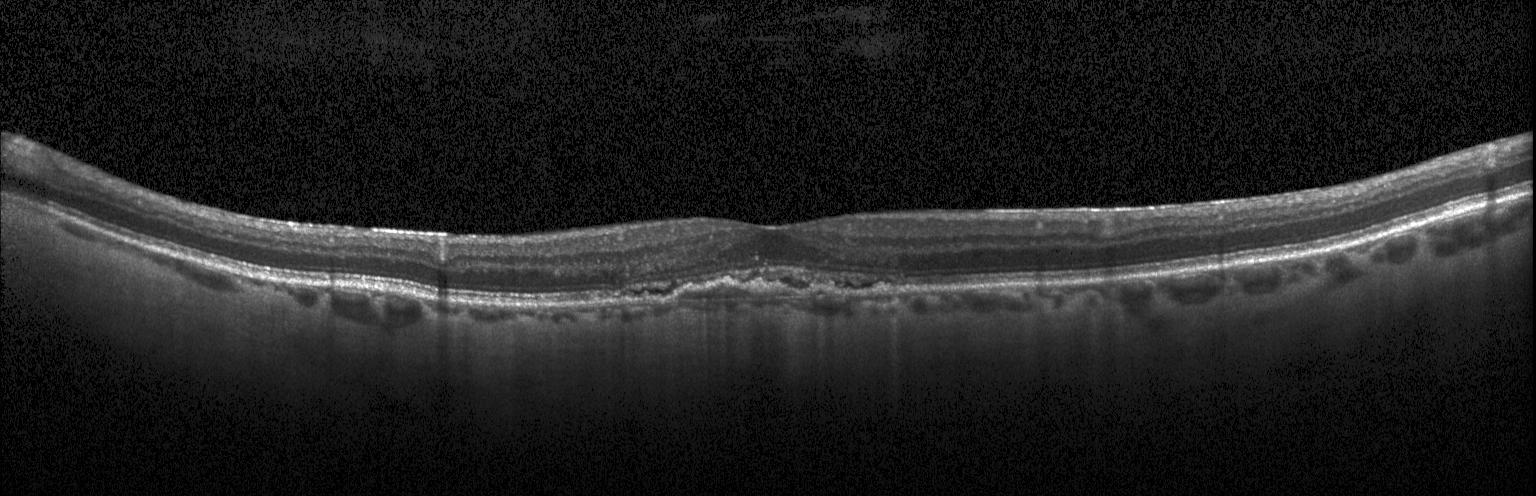 OCT line scan. Heidelberg Spectralis. SD-OCT. Diagnosis: choroidal neovascularization (CNV).